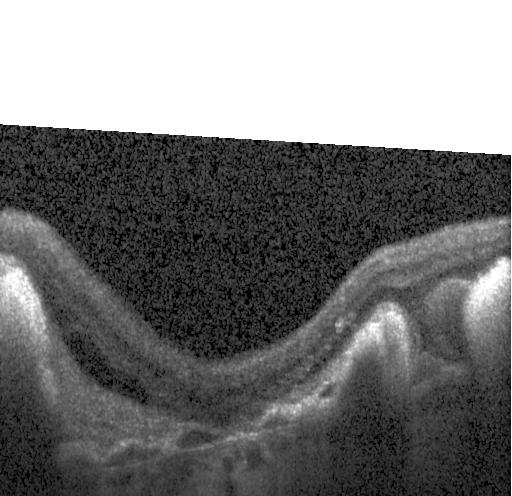
CNV.